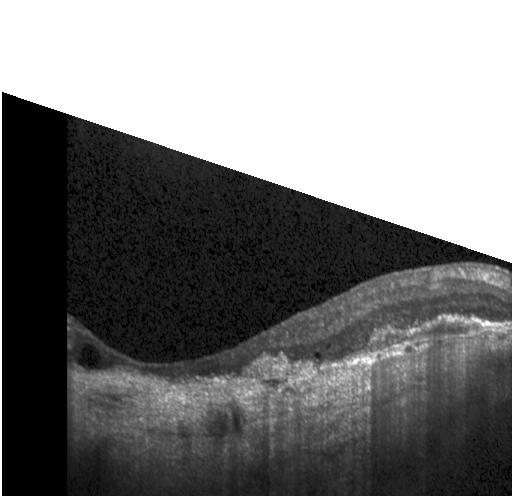 Heidelberg Spectralis; OCT B-scan; spectral-domain OCT
This B-scan demonstrates choroidal neovascularization (CNV).